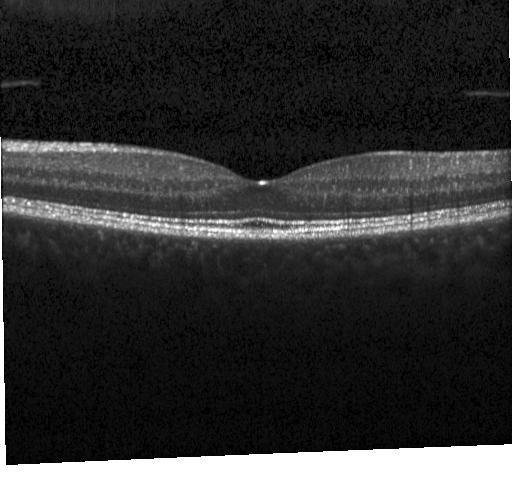

Assessment: no choroidal neovascularization, no diabetic macular edema, and no drusen.